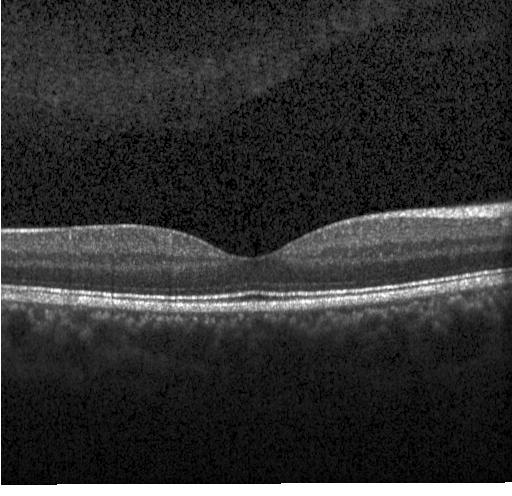
Retinal OCT B-scan; Heidelberg Spectralis; centered on the fovea. Diagnosis: neither choroidal neovascularization, diabetic macular edema, nor drusen.